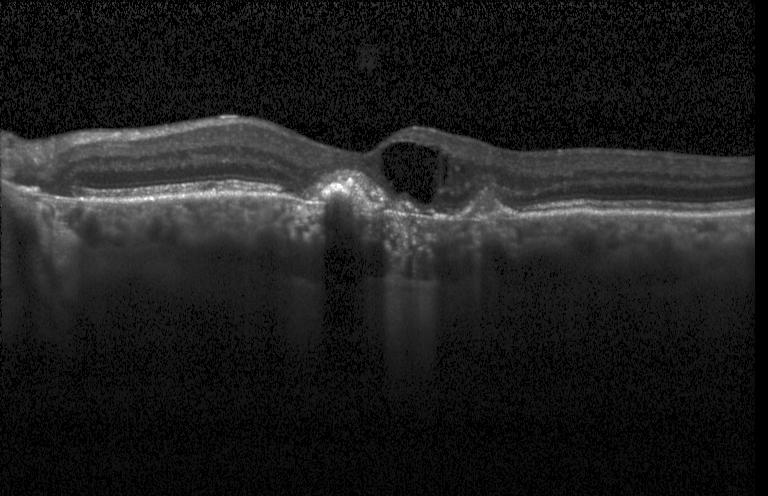 Retinal OCT B-scan, instrument: Heidelberg Spectralis, centered on the fovea, spectral-domain optical coherence tomography.
Dx: CNV.